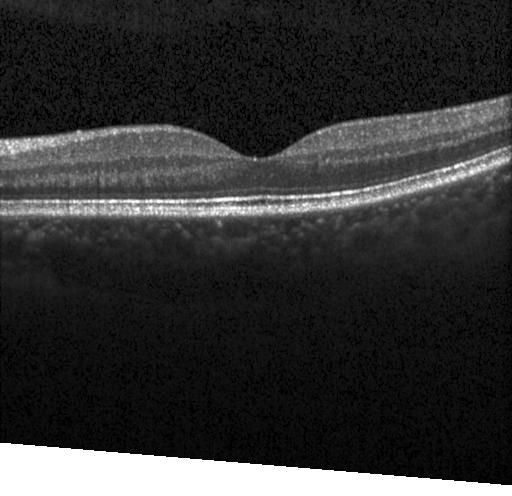 Centered on the fovea · optical coherence tomography B-scan · Heidelberg Spectralis OCT system · spectral-domain OCT. Diagnosis: no evidence of CNV, DME, or drusen.